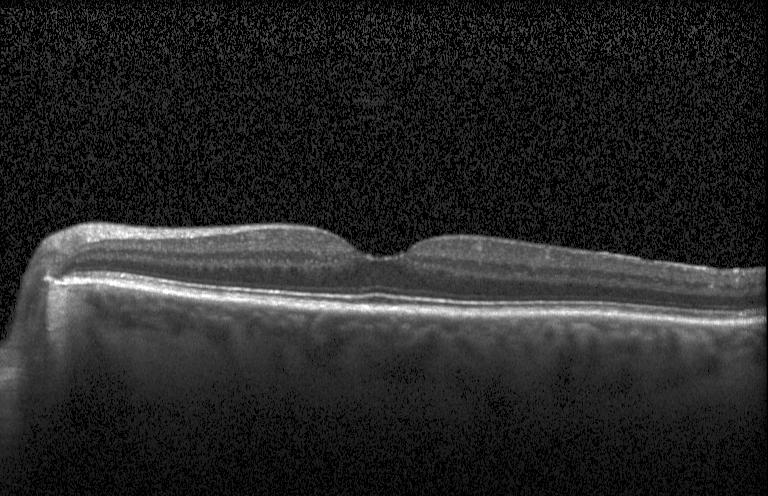 No CNV, DME, or drusen.